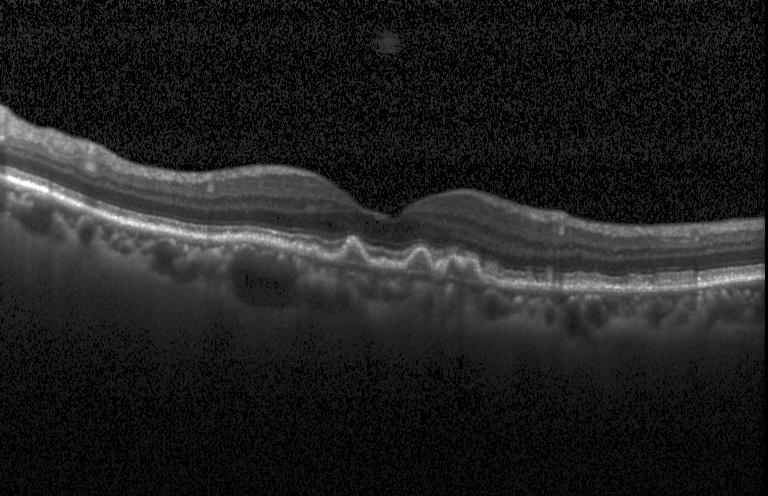

Impression: multiple drusen.